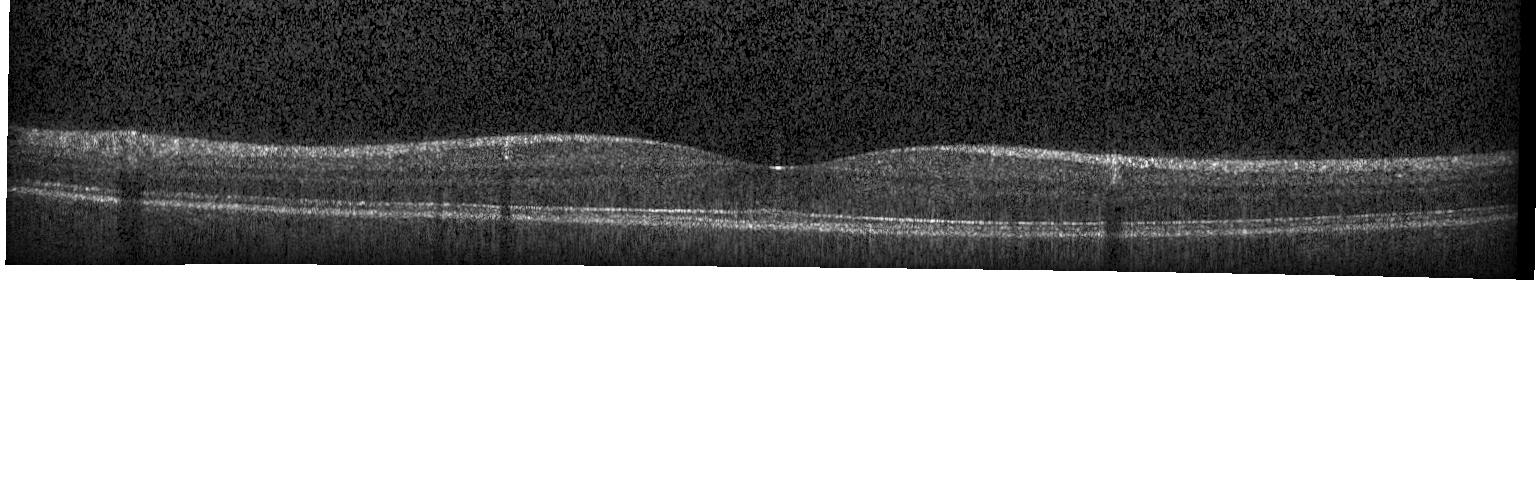
The scan shows neither CNV, DME, nor drusen.